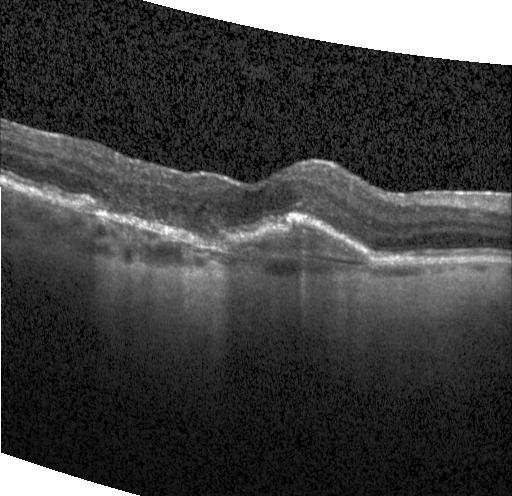
Macular OCT demonstrating choroidal neovascularization.